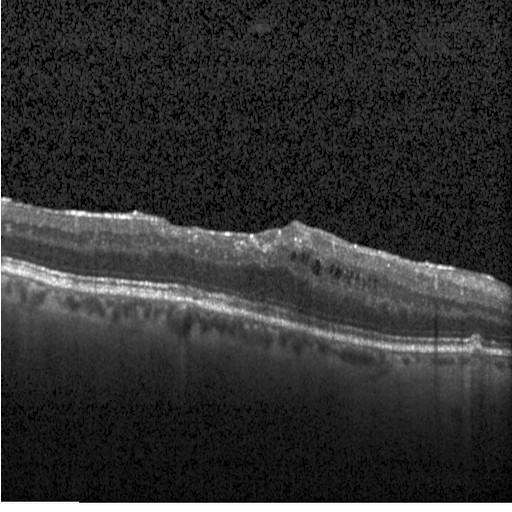
Retinal OCT cross-section showing diabetic macular edema.